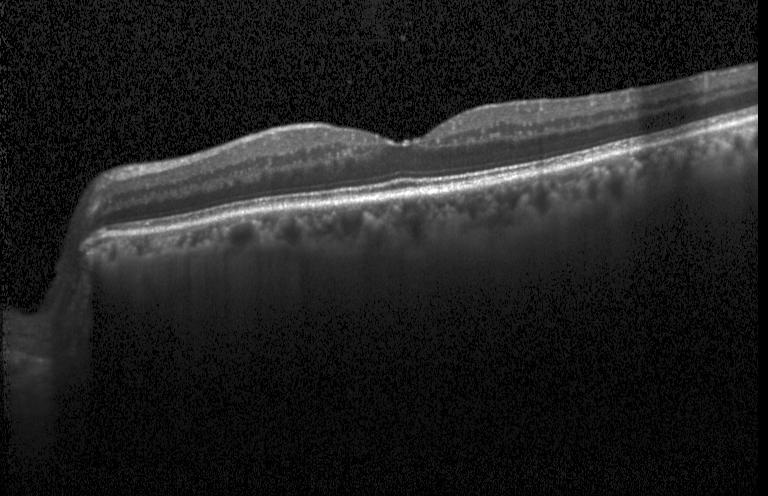
Horizontal scan through the fovea · OCT B-scan · spectral-domain optical coherence tomography · Heidelberg Spectralis OCT system. Finding: no choroidal neovascularization, no diabetic macular edema, and no drusen.